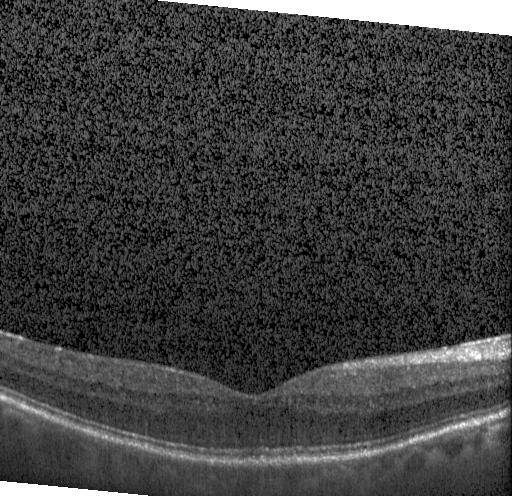

Finding: no evidence of choroidal neovascularization, diabetic macular edema, or drusen.